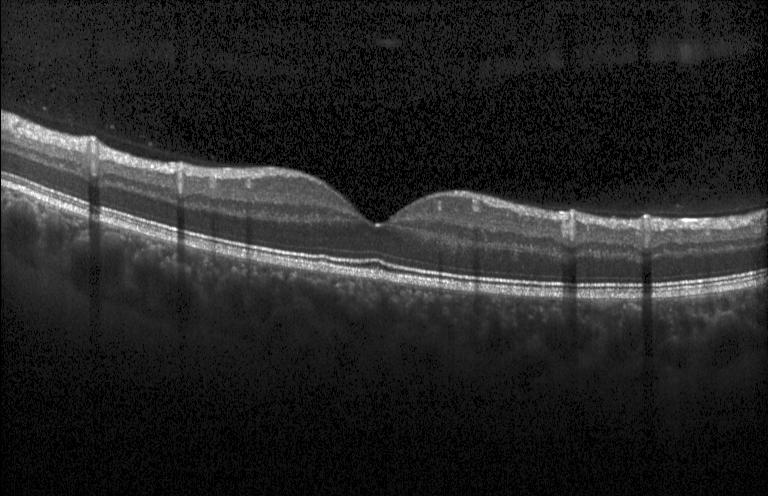 Finding: no choroidal neovascularization, no diabetic macular edema, and no drusen.